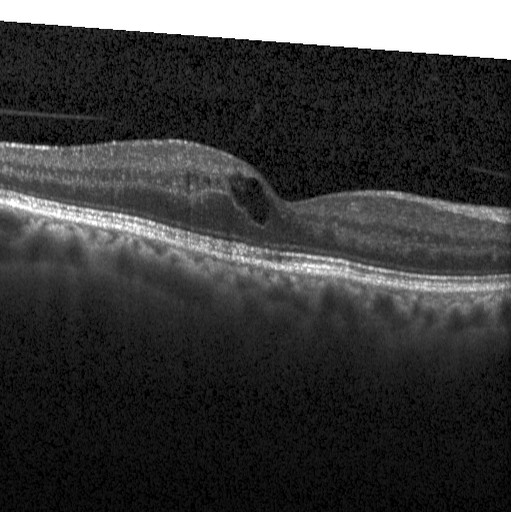
OCT finding: diabetic macular edema.